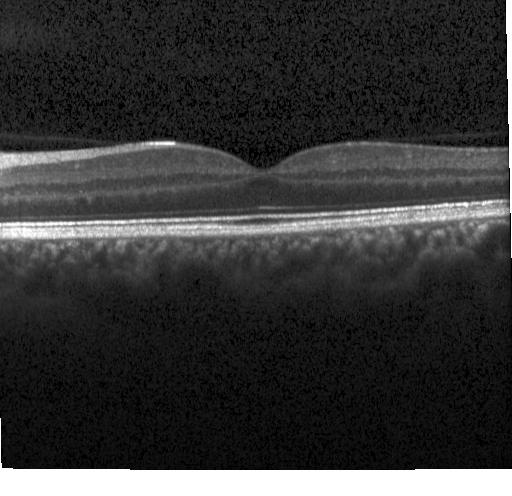

Retinal OCT B-scan. Acquired on a Heidelberg Spectralis. Spectral-domain OCT
OCT finding: no evidence of choroidal neovascularization, diabetic macular edema, or drusen.